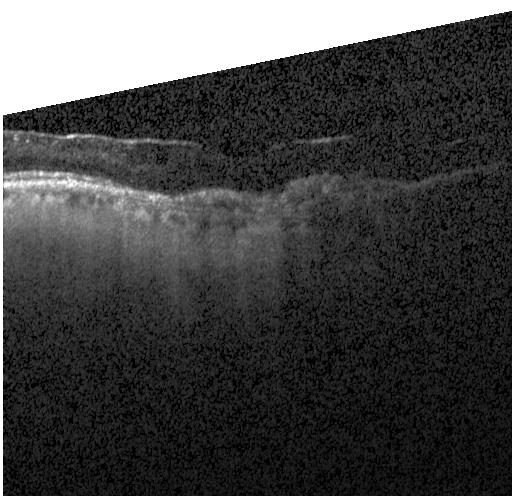 Spectral-domain OCT; horizontal scan through the fovea; retinal OCT B-scan
Macular OCT: a choroidal neovascular membrane.